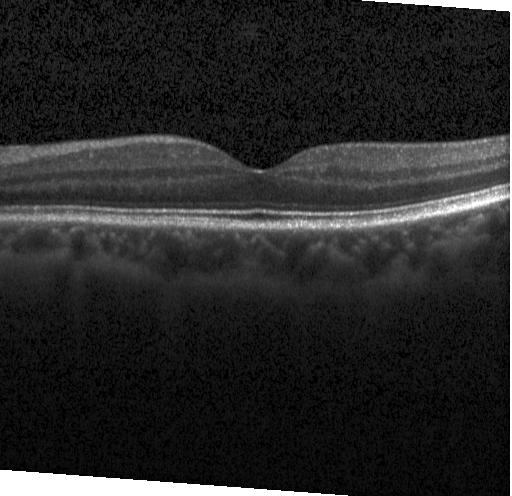

Retinal OCT cross-section
No choroidal neovascularization, no diabetic macular edema, and no drusen.